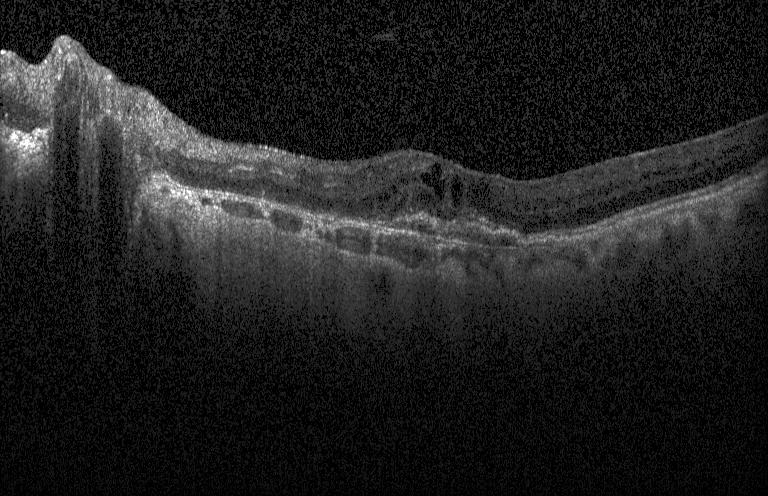
OCT B-scan. Diagnosis: a choroidal neovascular membrane.